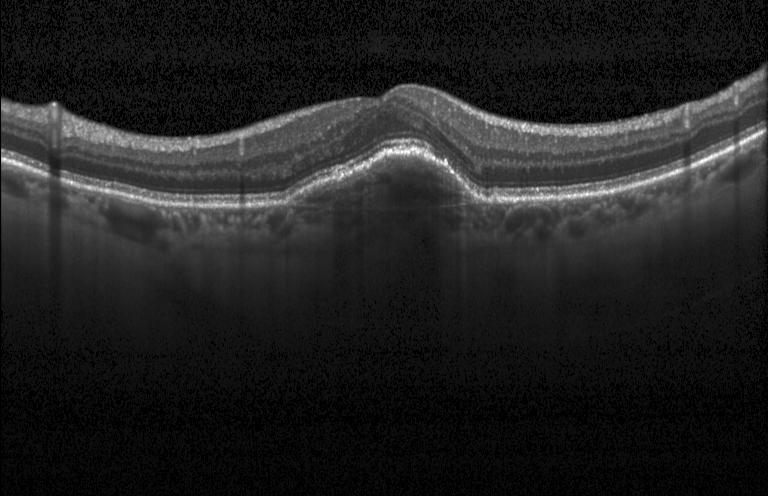 This B-scan demonstrates a choroidal neovascular membrane.